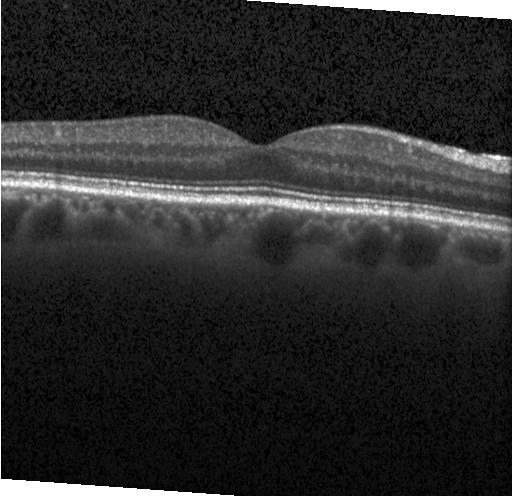

Impression: no choroidal neovascularization, diabetic macular edema, or drusen.